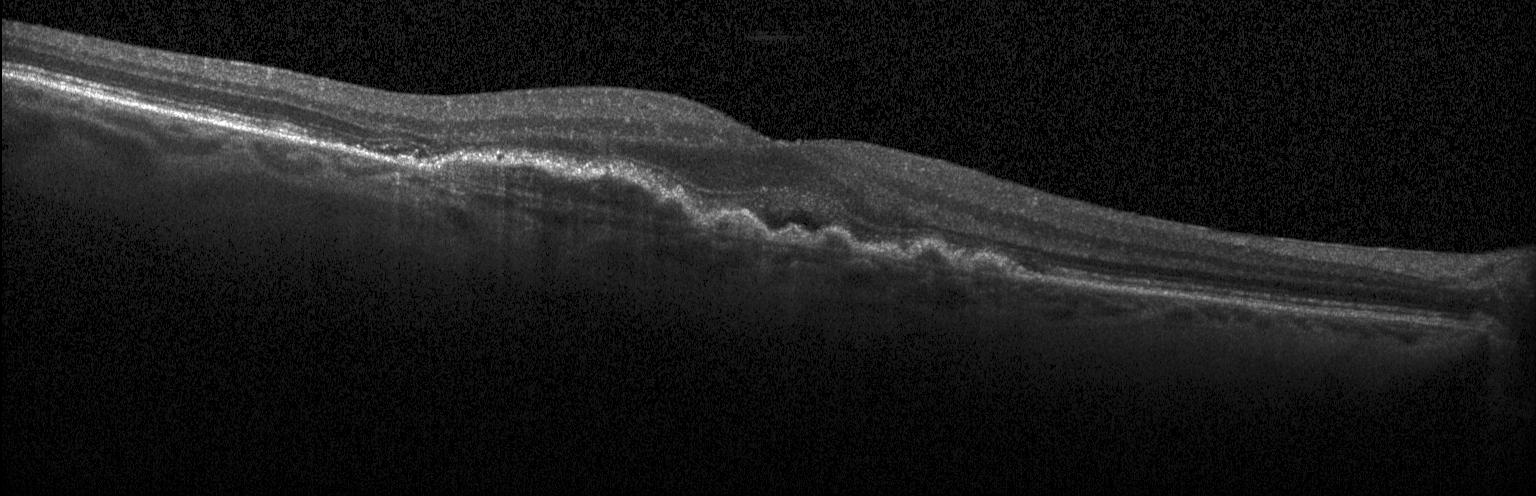 Spectral-domain optical coherence tomography; retinal OCT cross-section; fovea-centered; Heidelberg Spectralis OCT system
Finding: a choroidal neovascular membrane.